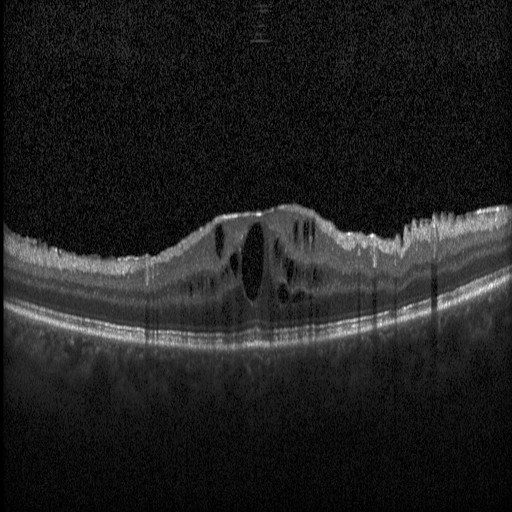 Finding: diabetic macular edema.